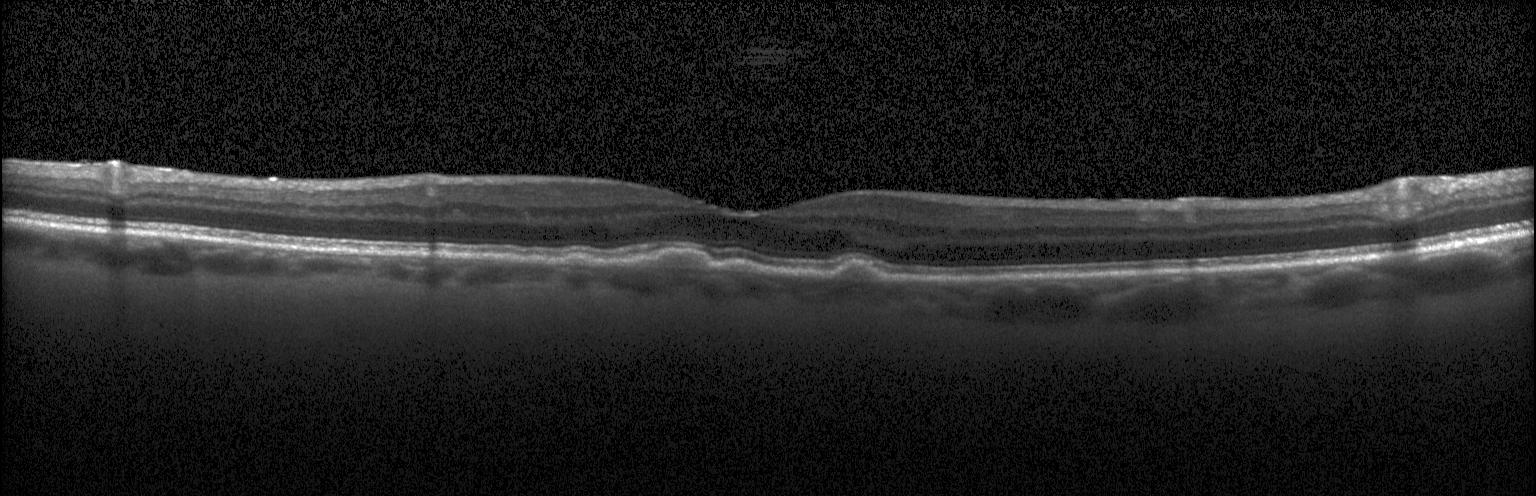 Optical coherence tomography scan. Heidelberg Spectralis. Spectral-domain OCT
Macular OCT: sub-RPE drusenoid deposits.